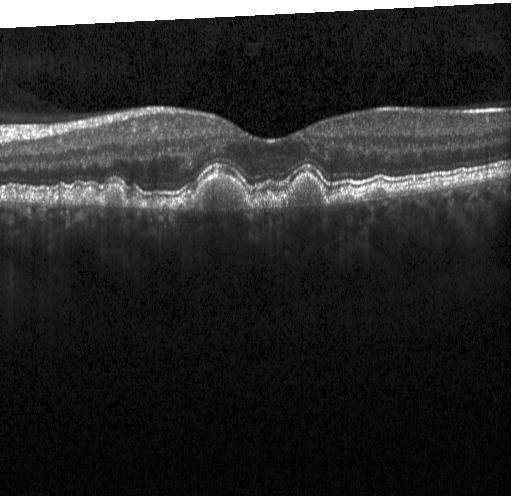 Retinal OCT B-scan — Diagnosis: drusen.